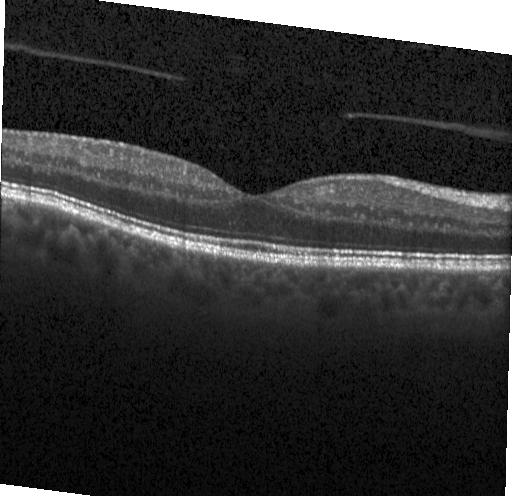

Macular scan; retinal OCT cross-section; SD-OCT; instrument: Heidelberg Spectralis
Impression: no CNV, no DME, and no drusen.